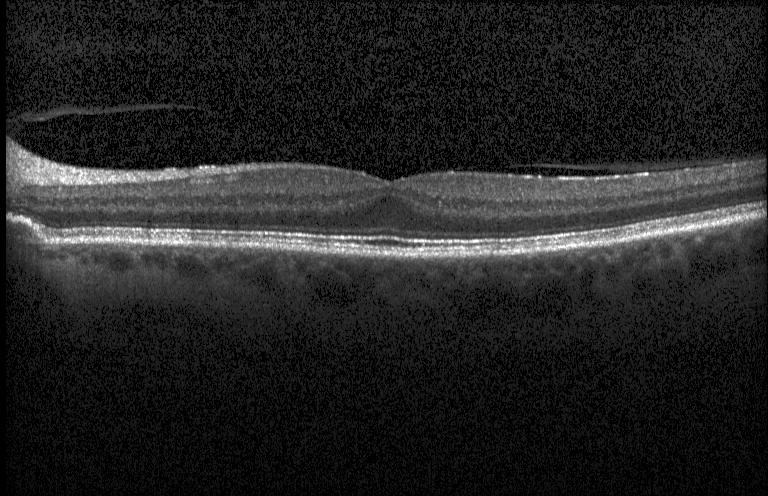
Retinal OCT B-scan — Finding: neither choroidal neovascularization, diabetic macular edema, nor drusen.